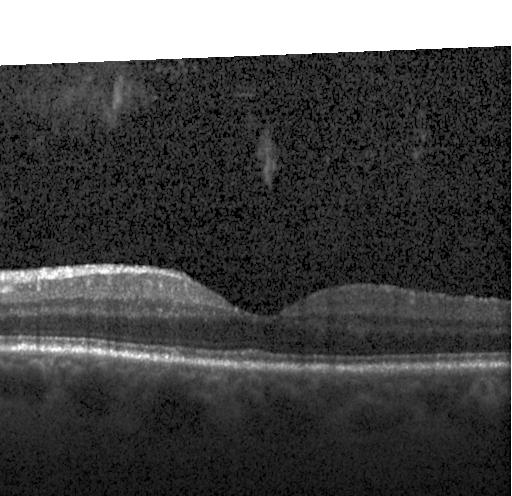

OCT B-scan showing neither CNV, DME, nor drusen.